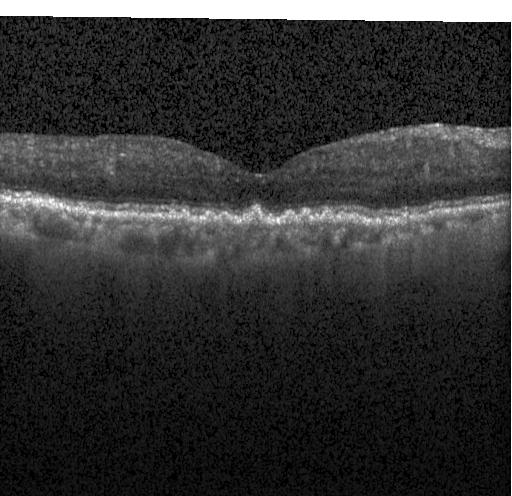
Dx: drusen.